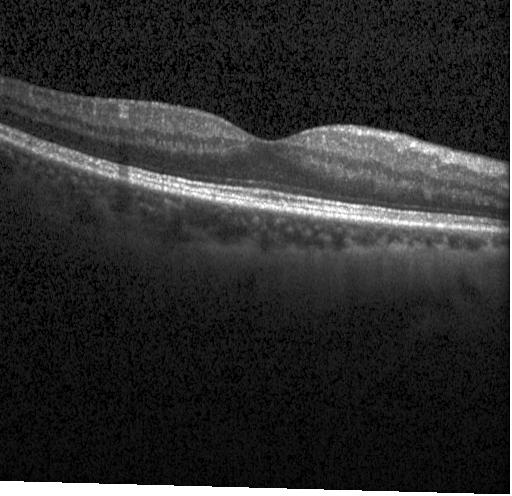 SD-OCT; OCT line scan; through the macula; instrument: Heidelberg Spectralis
This B-scan demonstrates no choroidal neovascularization, no diabetic macular edema, and no drusen.